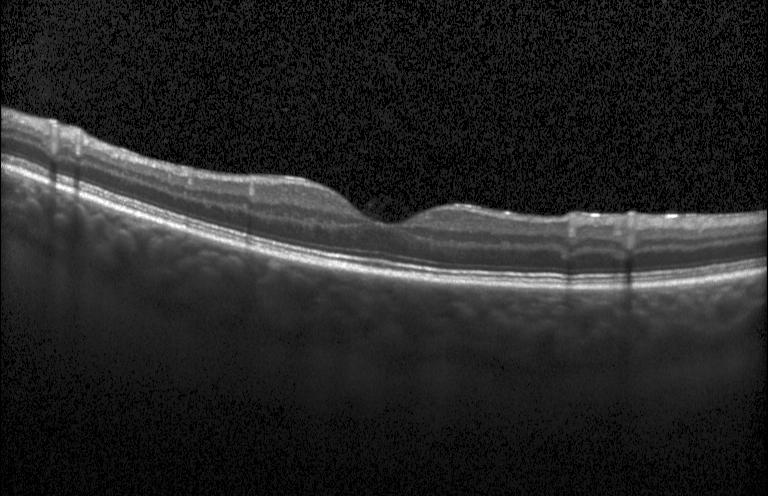
Instrument: Heidelberg Spectralis; OCT B-scan; SD-OCT.
Diagnosis: no evidence of CNV, DME, or drusen.